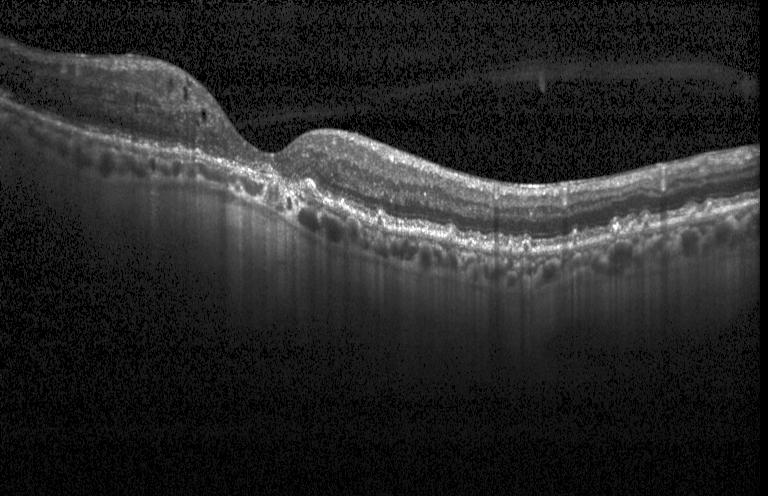 Fovea-centered, spectral-domain optical coherence tomography, Heidelberg Spectralis, retinal OCT cross-section — Diagnosis: choroidal neovascularization.